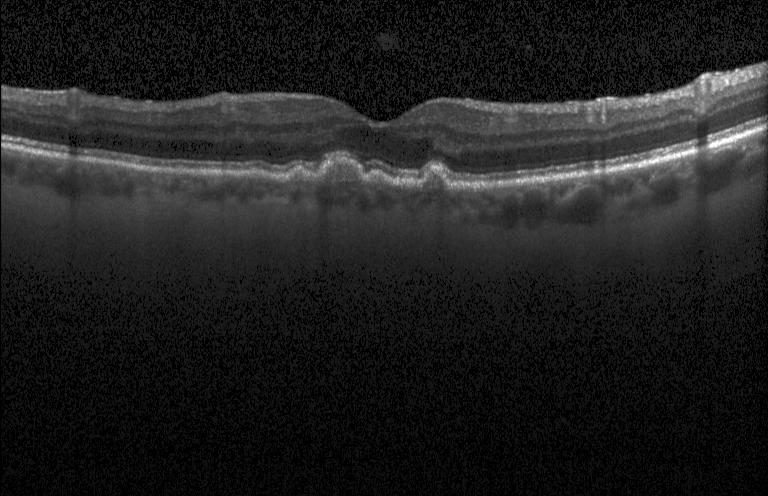
SD-OCT, centered on the fovea, retinal OCT B-scan, Heidelberg Spectralis — OCT finding: drusen.